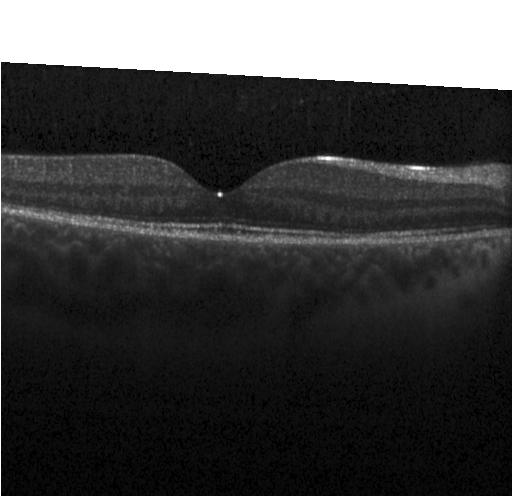

No CNV, no DME, and no drusen.